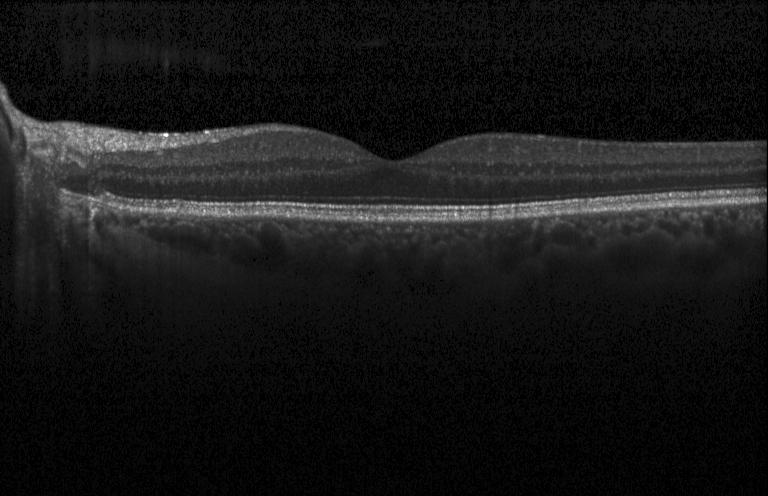 No evidence of choroidal neovascularization, diabetic macular edema, or drusen.